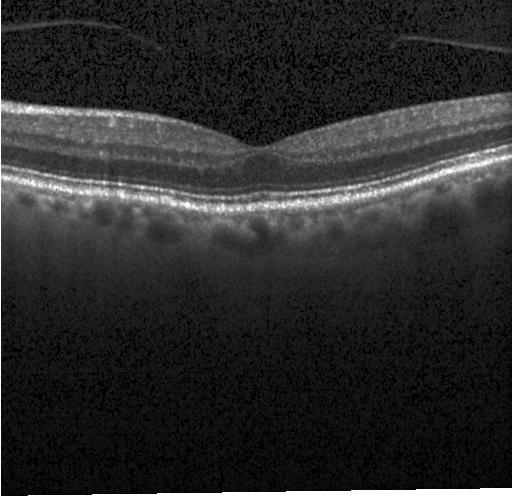

Retinal OCT B-scan; SD-OCT.
OCT finding: no choroidal neovascularization, no diabetic macular edema, and no drusen.